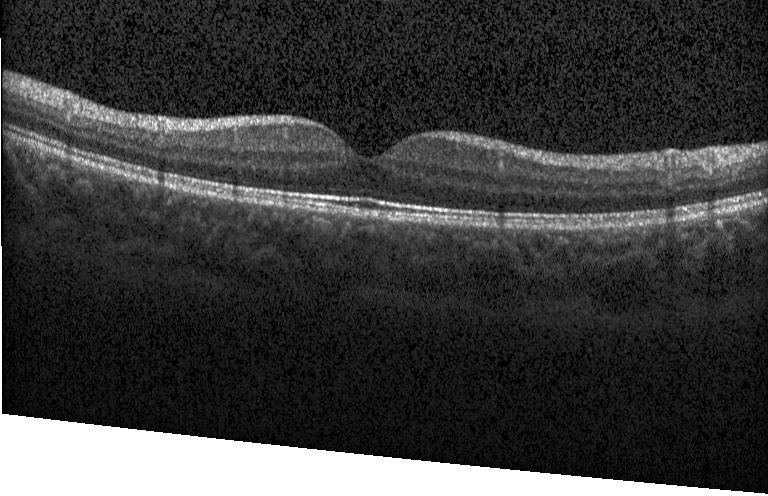 Optical coherence tomography scan — Impression: neither choroidal neovascularization, diabetic macular edema, nor drusen.